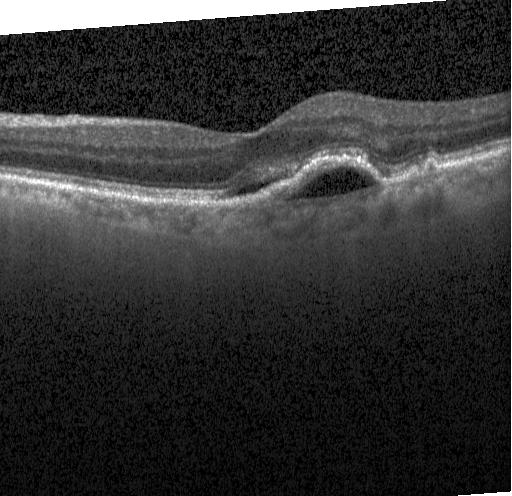

Spectral-domain OCT. OCT B-scan. Horizontal scan through the fovea. Heidelberg Spectralis OCT system.
The scan shows choroidal neovascularization.